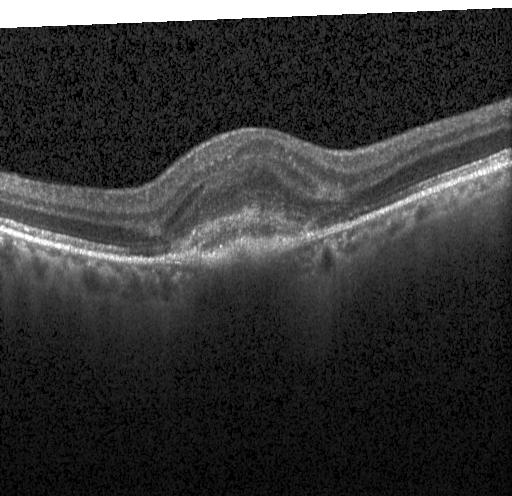

Retinal OCT cross-section
Diagnosis: choroidal neovascularization.